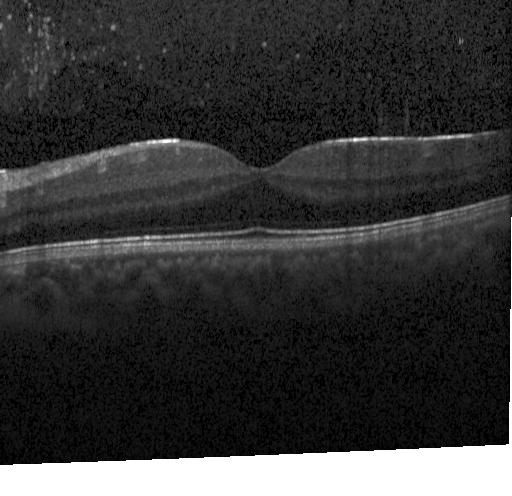

Optical coherence tomography B-scan; acquired on a Heidelberg Spectralis; spectral-domain optical coherence tomography; through the macula. Assessment: no CNV, DME, or drusen.